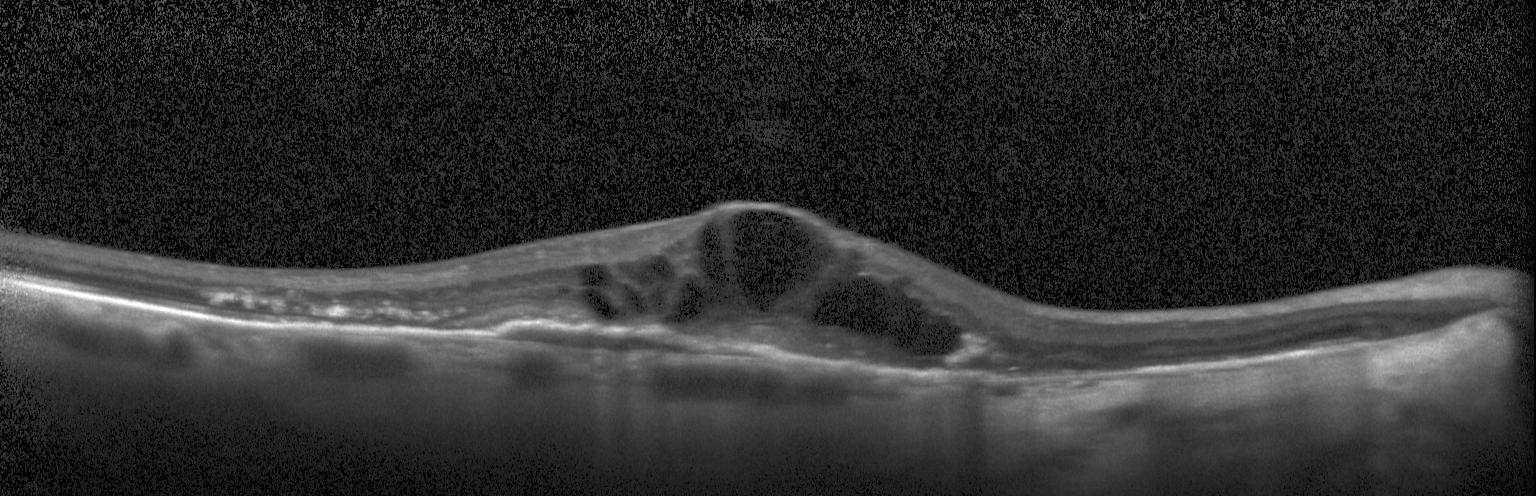

Dx: choroidal neovascularization.